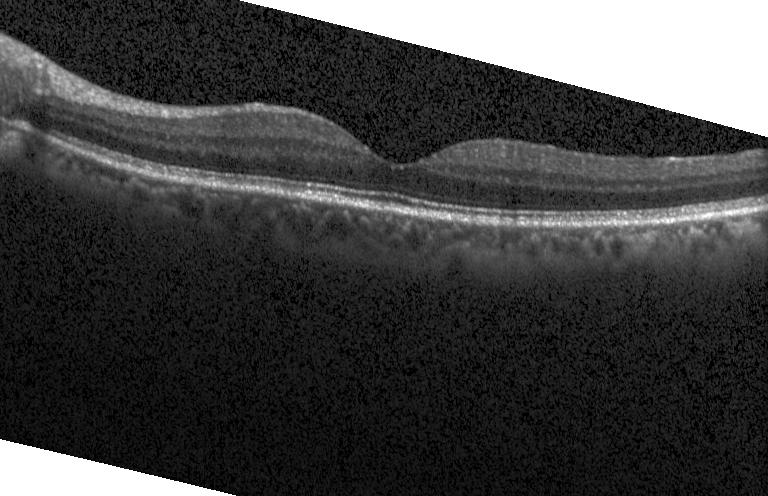 OCT B-scan. Horizontal scan through the fovea — Macular OCT: no choroidal neovascularization, no diabetic macular edema, and no drusen.